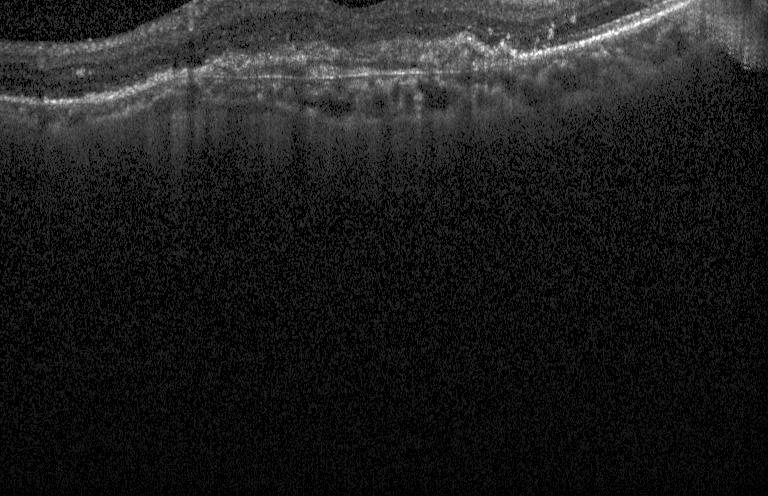 Impression: a choroidal neovascular membrane.